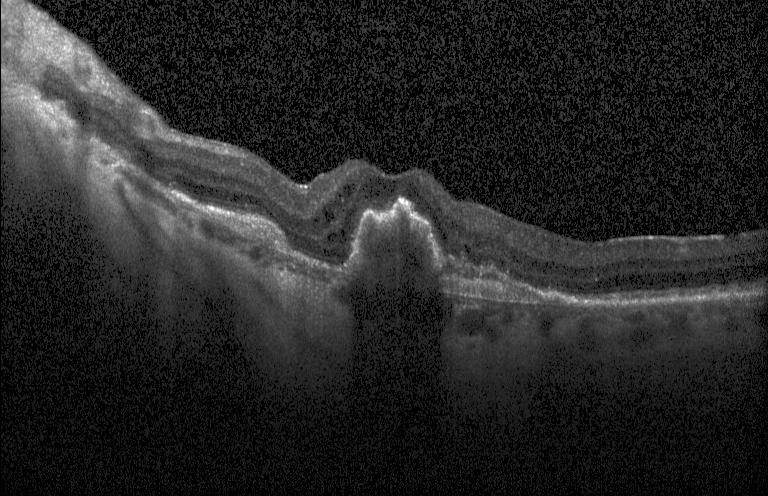 Optical coherence tomography B-scan
Macular OCT: choroidal neovascularization.